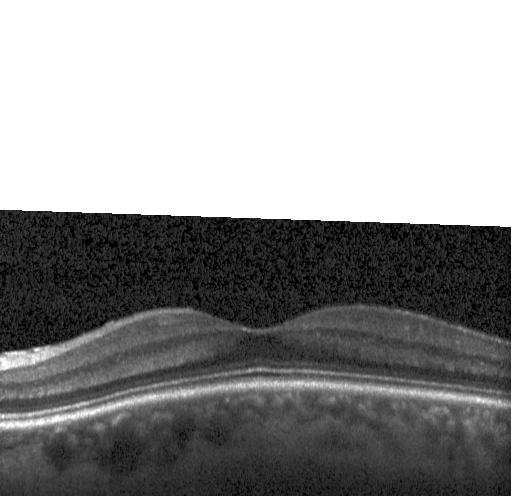
Spectral-domain optical coherence tomography · retinal OCT cross-section · through the macula · instrument: Heidelberg Spectralis
Diagnosis: no CNV, DME, or drusen.